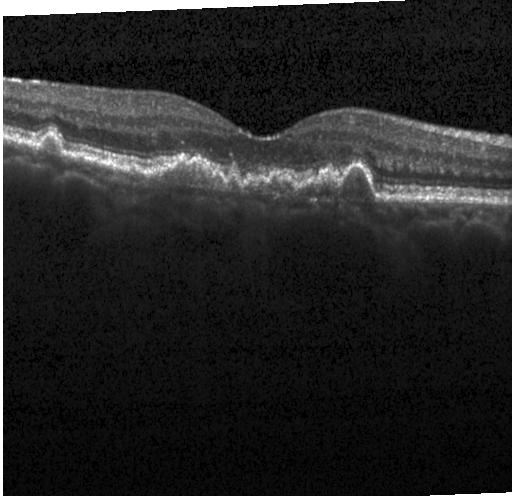 Fovea-centered, Heidelberg Spectralis, optical coherence tomography scan.
Dx: multiple drusen.